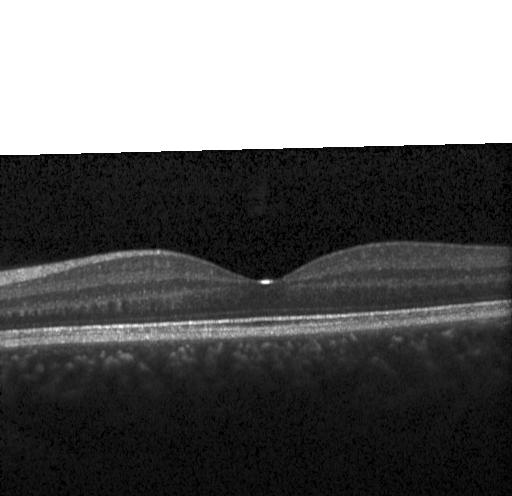

Horizontal scan through the fovea · OCT line scan.
Finding: neither choroidal neovascularization, diabetic macular edema, nor drusen.